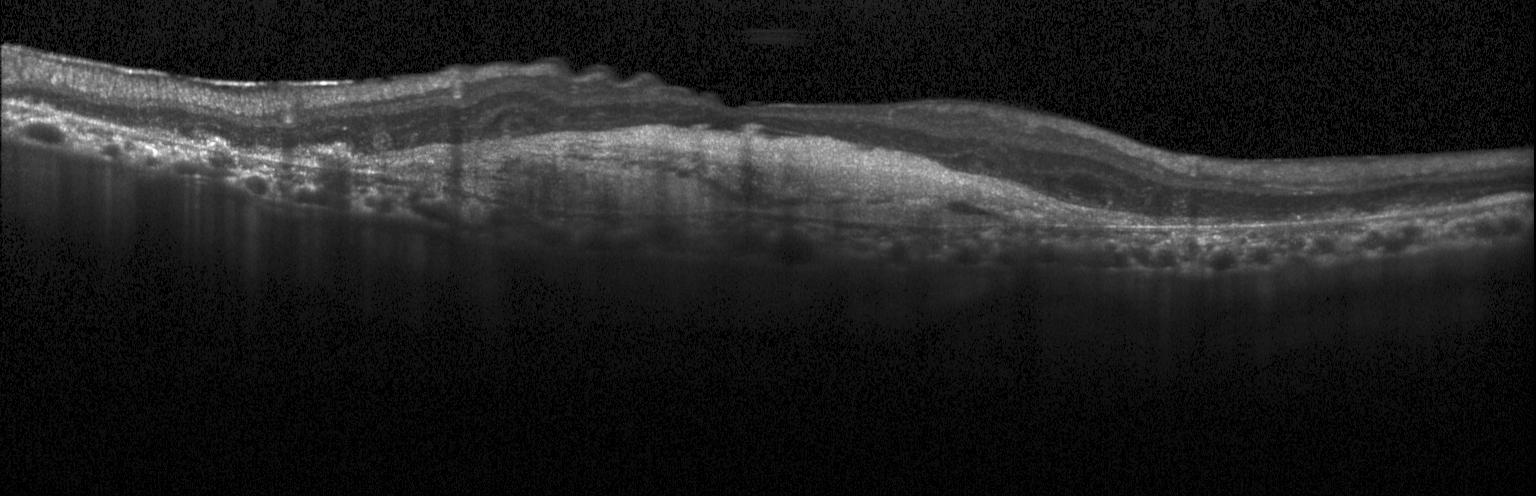
OCT B-scan · centered on the fovea · spectral-domain OCT · acquired on a Heidelberg Spectralis.
Impression: a choroidal neovascular membrane.